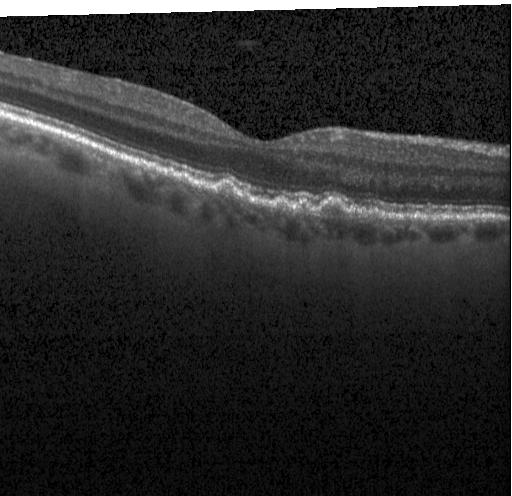

Heidelberg Spectralis OCT system. Optical coherence tomography B-scan. Fovea-centered.
Diagnosis: multiple drusen.